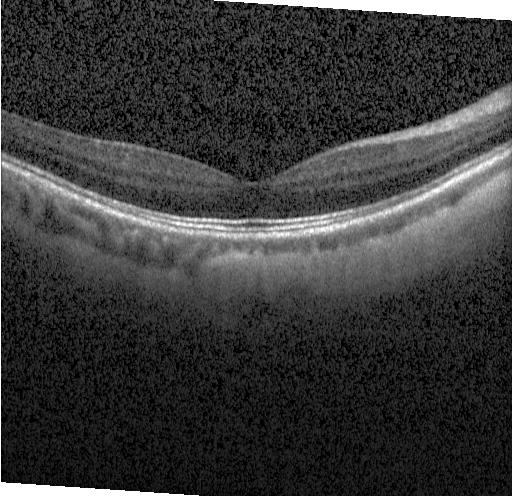

OCT B-scan.
Assessment: no evidence of choroidal neovascularization, diabetic macular edema, or drusen.